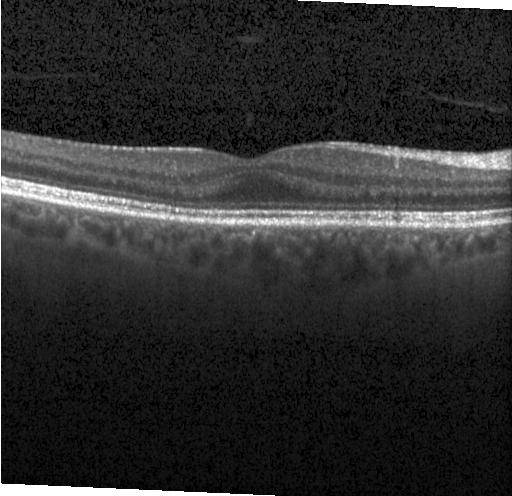

Acquired on a Heidelberg Spectralis. OCT line scan. Finding: no choroidal neovascularization, diabetic macular edema, or drusen.